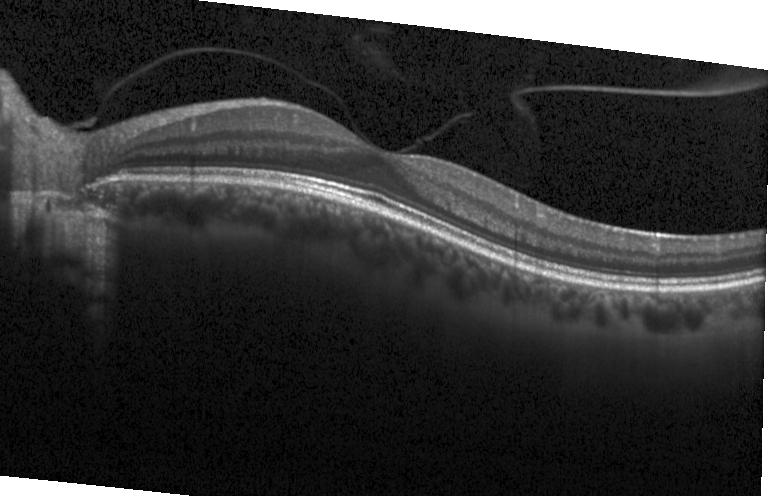

Heidelberg Spectralis OCT system; retinal OCT B-scan; horizontal scan through the fovea — This B-scan demonstrates no choroidal neovascularization, no diabetic macular edema, and no drusen.